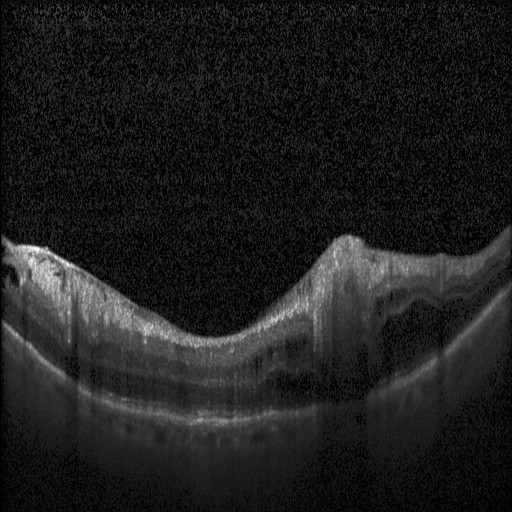
Optical coherence tomography B-scan. Through the macula. Spectral-domain optical coherence tomography. Acquired on a Heidelberg Spectralis. Macular OCT: DME.